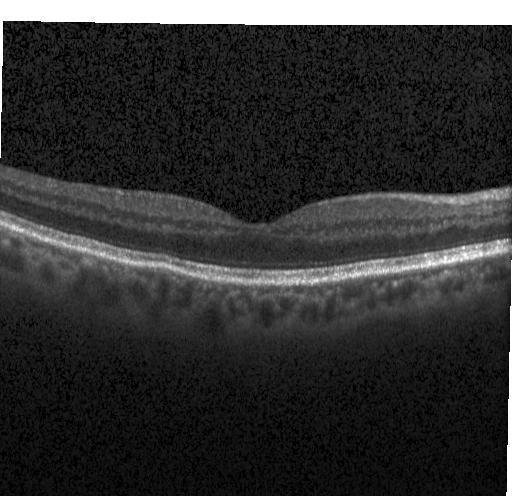 Assessment: no CNV, no DME, and no drusen.